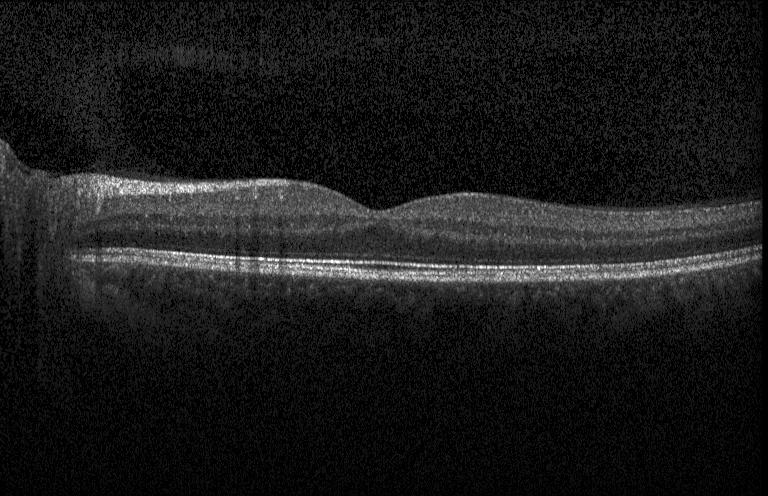 Dx: neither choroidal neovascularization, diabetic macular edema, nor drusen.